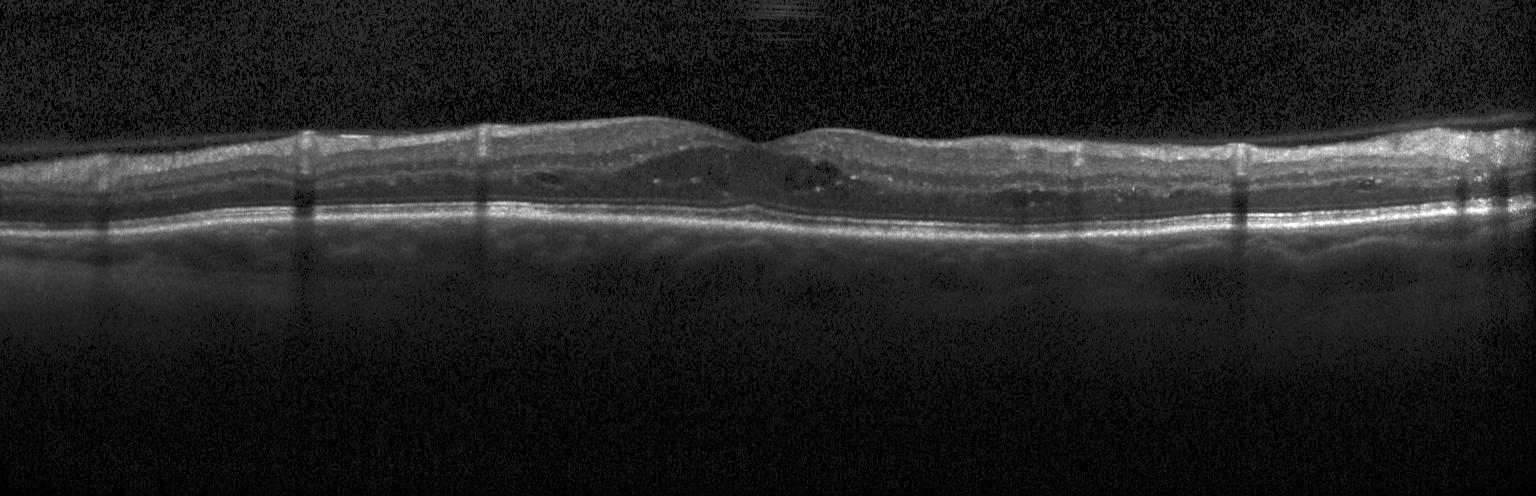

OCT line scan · Heidelberg Spectralis · SD-OCT · through the macula — Impression: DME.